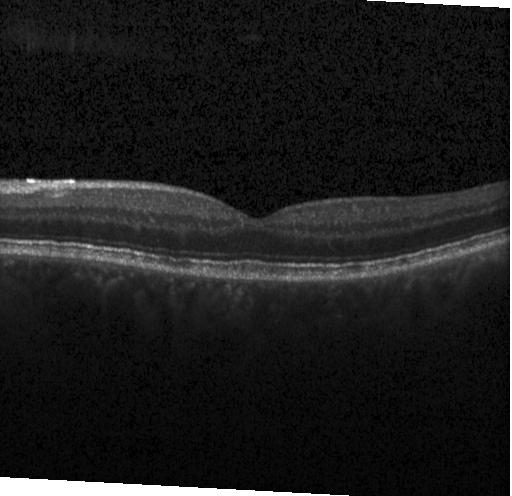 Horizontal scan through the fovea; optical coherence tomography B-scan; Heidelberg Spectralis.
Diagnosis: no evidence of CNV, DME, or drusen.